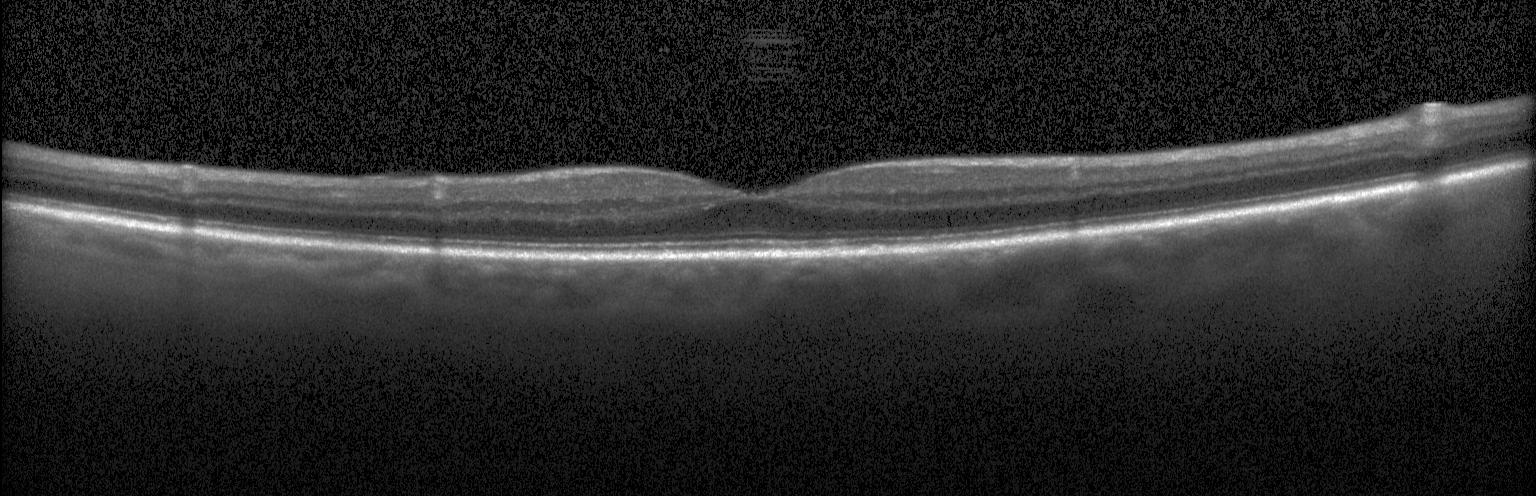 Spectral-domain optical coherence tomography, retinal OCT B-scan — Impression: no choroidal neovascularization, diabetic macular edema, or drusen.